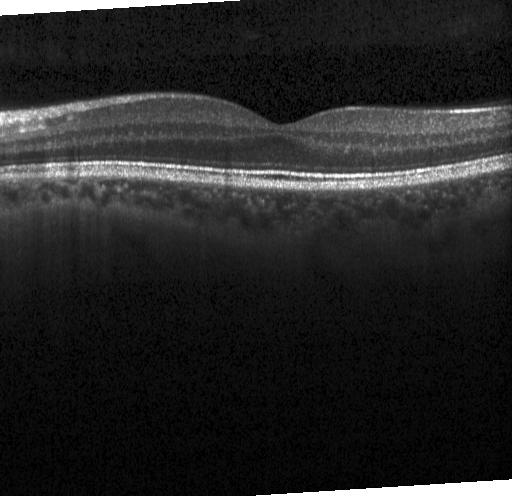 Optical coherence tomography scan
Diagnosis: no evidence of CNV, DME, or drusen.